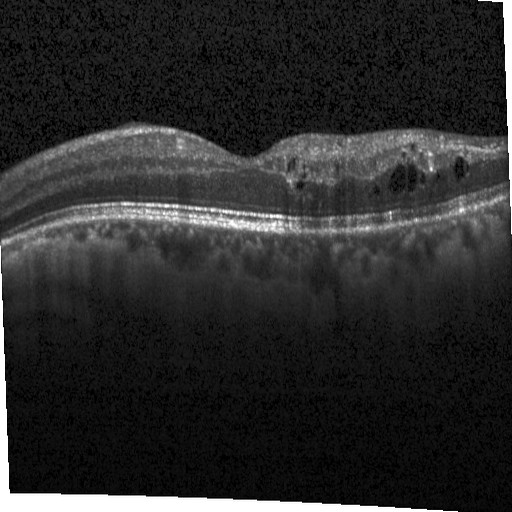

This B-scan demonstrates diabetic macular edema.